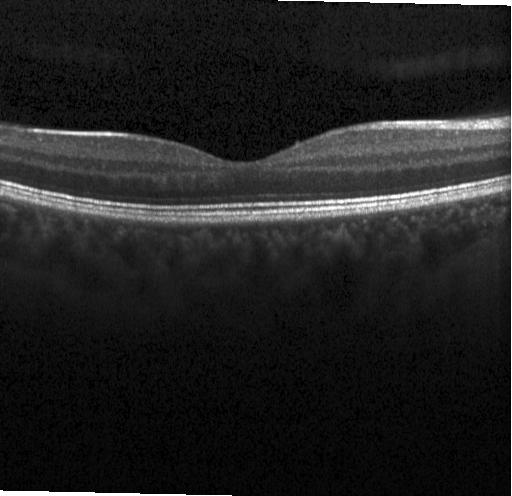
The scan shows neither CNV, DME, nor drusen.